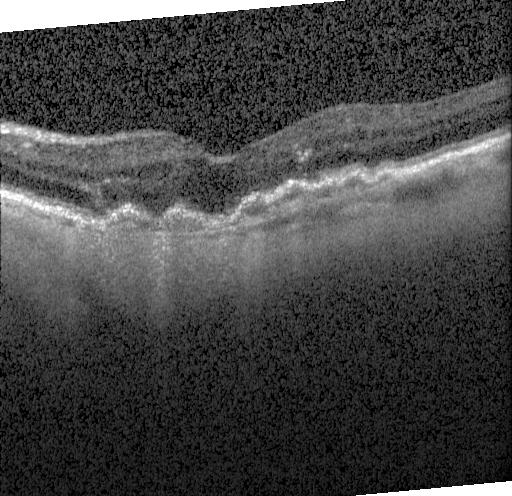 Retinal OCT cross-section showing a choroidal neovascular membrane.